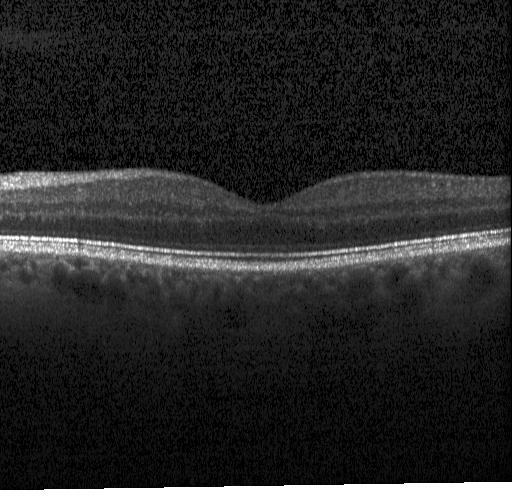 Optical coherence tomography scan — The scan shows neither CNV, DME, nor drusen.